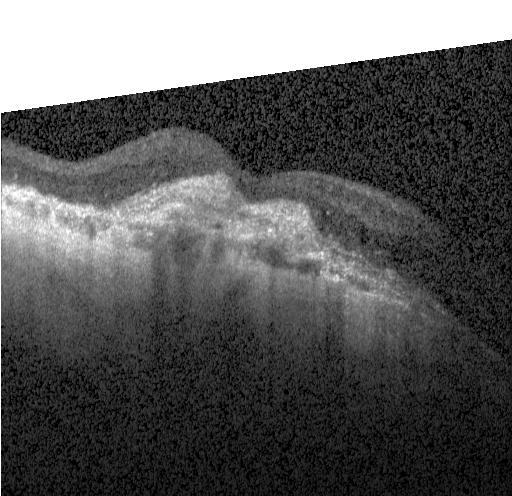

OCT B-scan
Choroidal neovascularization.